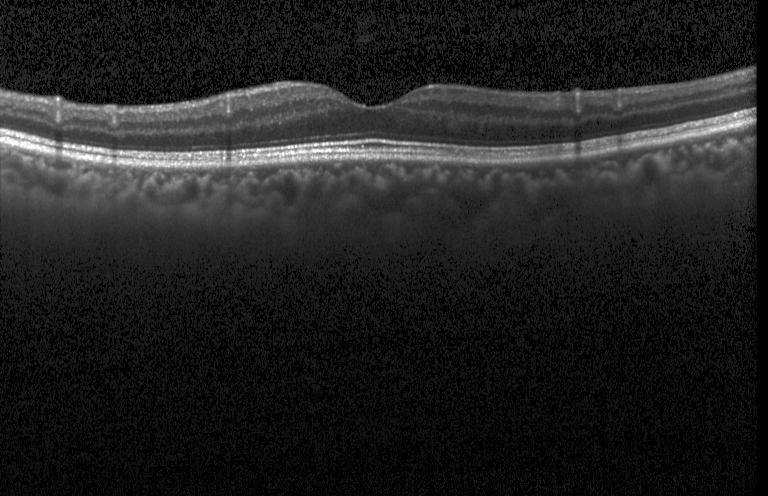
Retinal OCT cross-section. Spectral-domain OCT. Instrument: Heidelberg Spectralis. Through the macula — Assessment: no choroidal neovascularization, diabetic macular edema, or drusen.